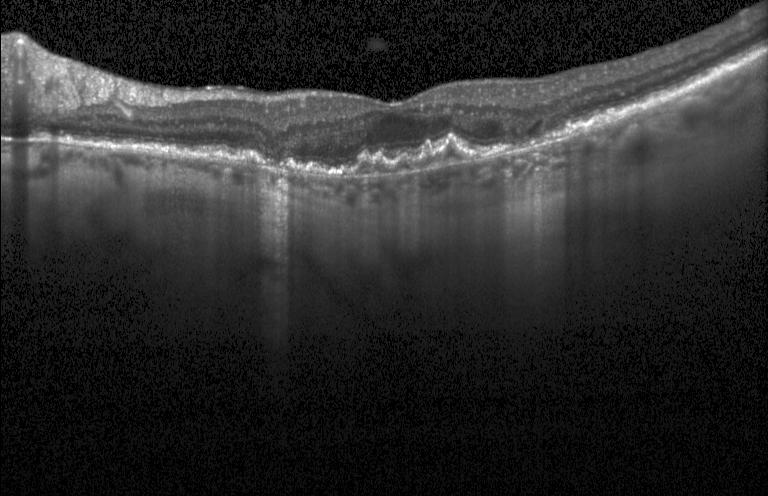 Finding: CNV.